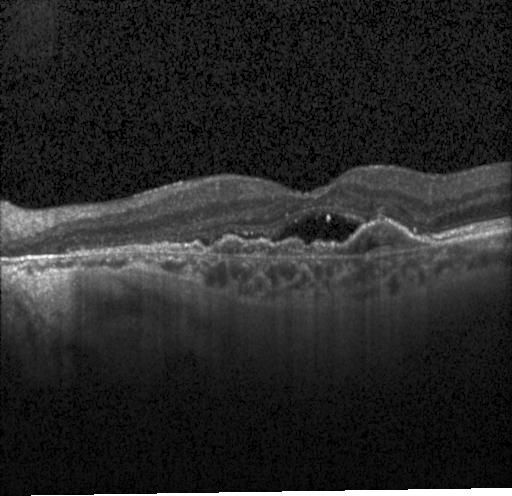 Acquired on a Heidelberg Spectralis · through the macula · OCT line scan
A choroidal neovascular membrane.